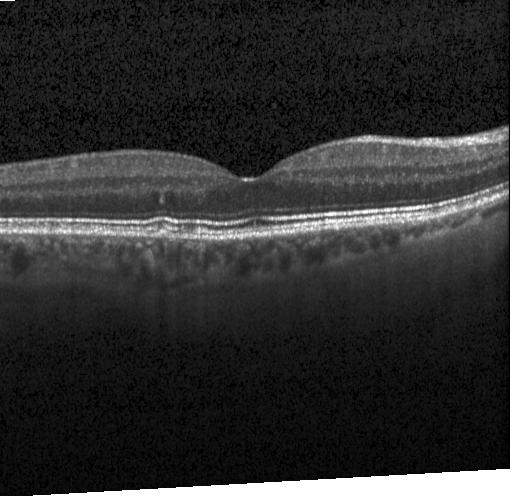 Retinal OCT B-scan · Heidelberg Spectralis · fovea-centered · SD-OCT
Finding: multiple drusen.